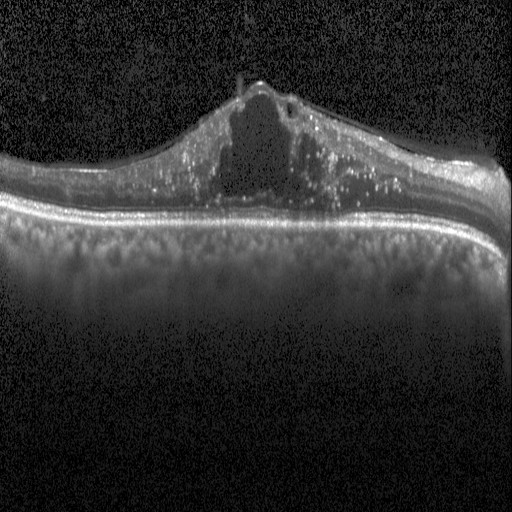 OCT line scan. Impression: diabetic macular edema (DME).